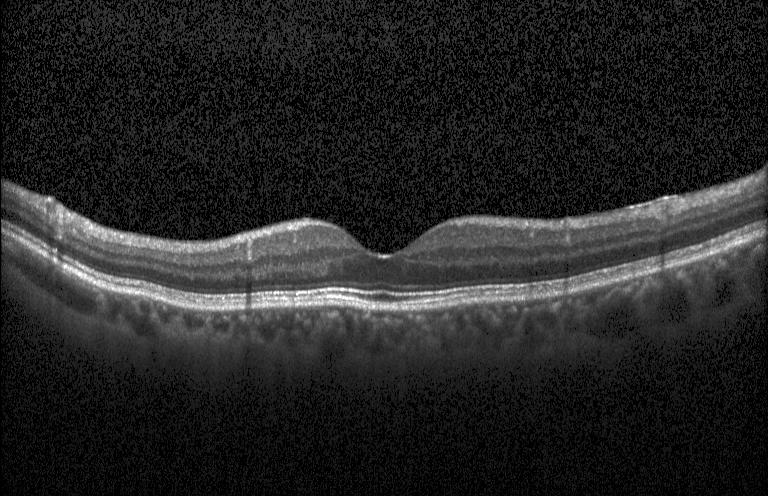

OCT B-scan showing neither choroidal neovascularization, diabetic macular edema, nor drusen.